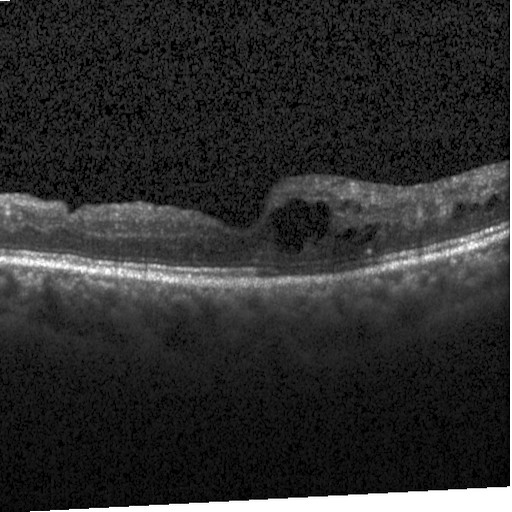

Diagnosis: diabetic macular edema (DME).